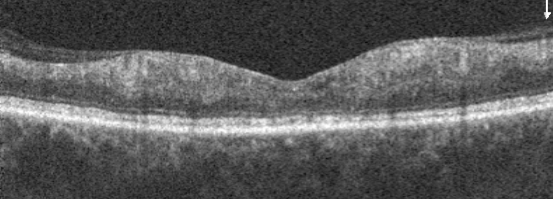
Retinal OCT B-scan. Fovea-centered.
Macular OCT: diabetic macular edema.